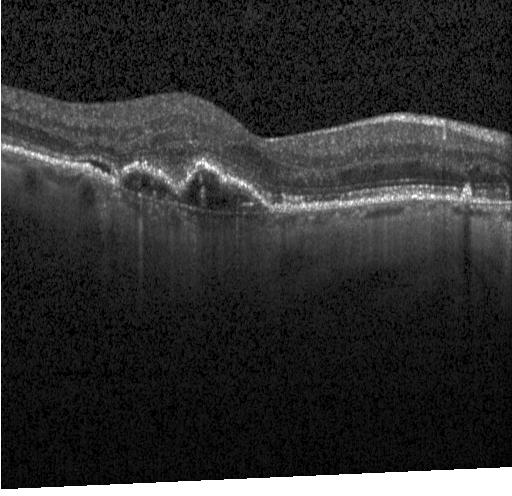
Spectral-domain optical coherence tomography · OCT line scan · through the macula. This B-scan demonstrates a choroidal neovascular membrane.